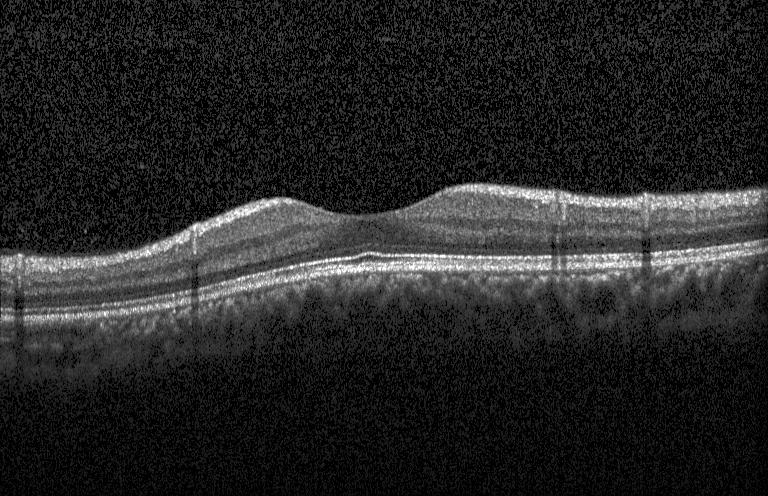
Spectral-domain optical coherence tomography · instrument: Heidelberg Spectralis · retinal OCT B-scan · fovea-centered. Assessment: no choroidal neovascularization, no diabetic macular edema, and no drusen.